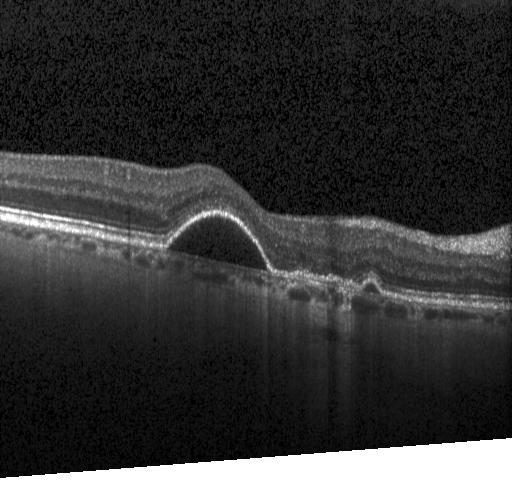
Acquired on a Heidelberg Spectralis. Spectral-domain optical coherence tomography. OCT B-scan.
The scan shows a choroidal neovascular membrane.